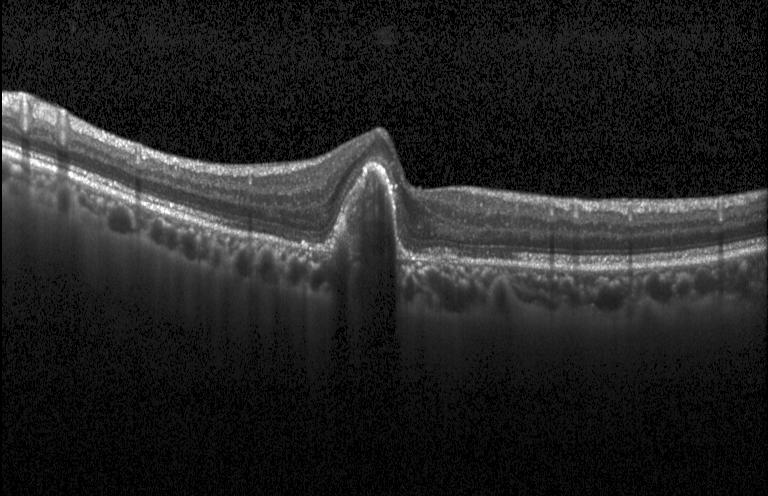
Retinal OCT B-scan. Macular OCT: choroidal neovascularization.